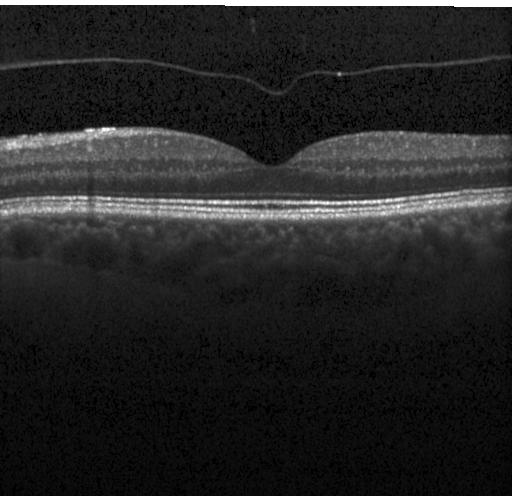 Impression: no CNV, no DME, and no drusen.